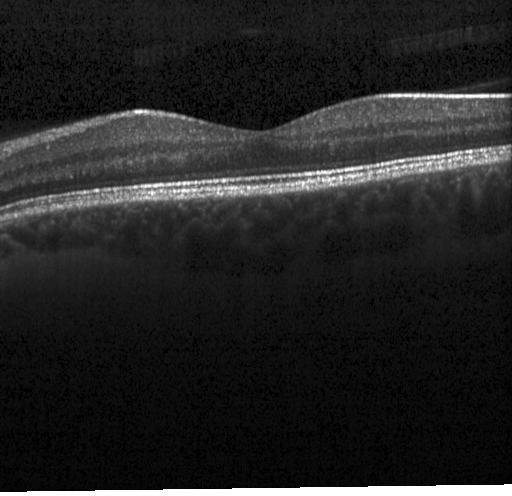

OCT finding: neither choroidal neovascularization, diabetic macular edema, nor drusen.